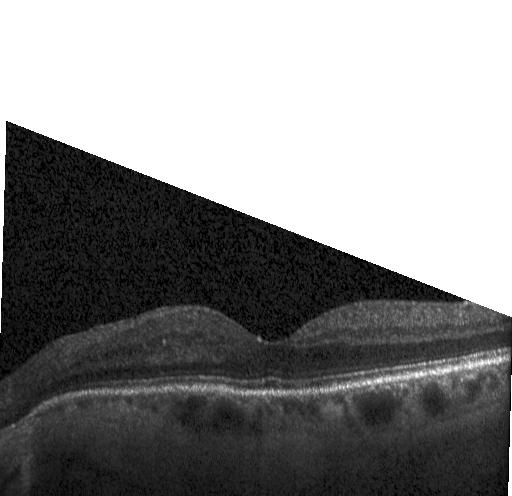
OCT B-scan.
Impression: neither choroidal neovascularization, diabetic macular edema, nor drusen.